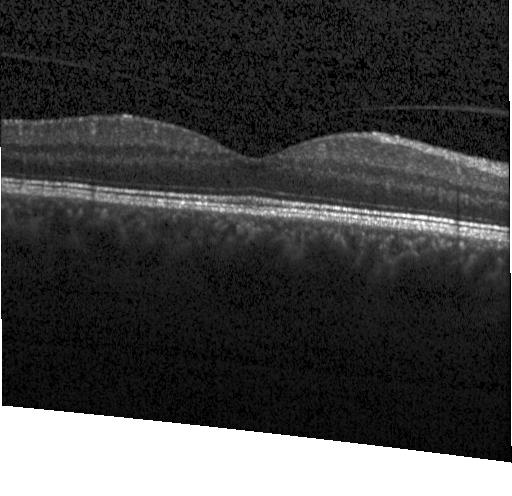 OCT B-scan showing no choroidal neovascularization, no diabetic macular edema, and no drusen.